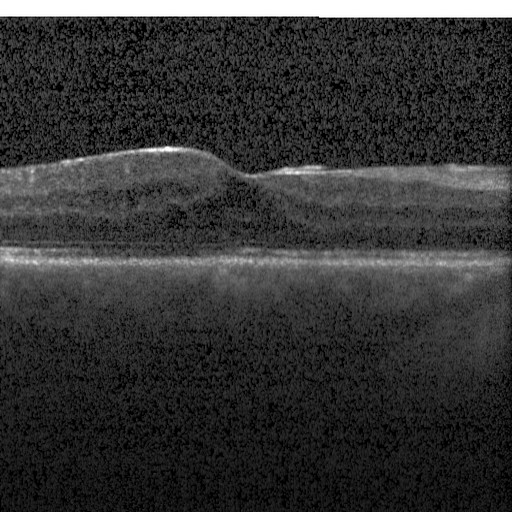
Retinal OCT B-scan, through the macula
Finding: diabetic macular edema.